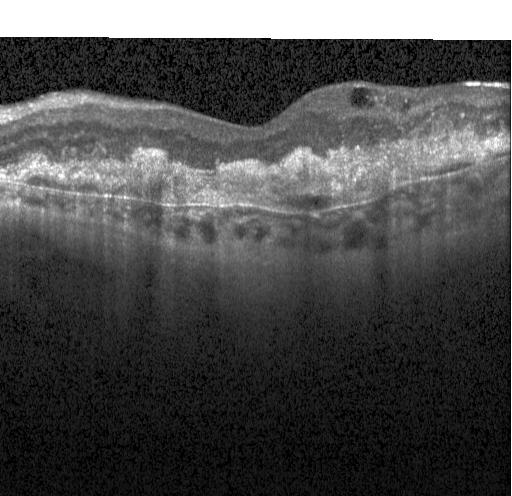 Macular scan, OCT line scan, acquired on a Heidelberg Spectralis, SD-OCT.
Diagnosis: a choroidal neovascular membrane.